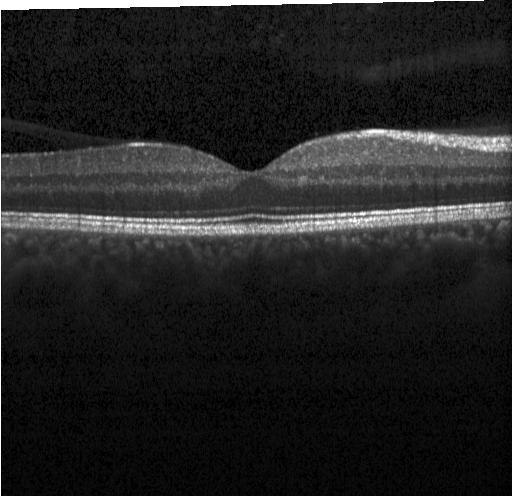 Retinal OCT cross-section, SD-OCT — Finding: neither choroidal neovascularization, diabetic macular edema, nor drusen.